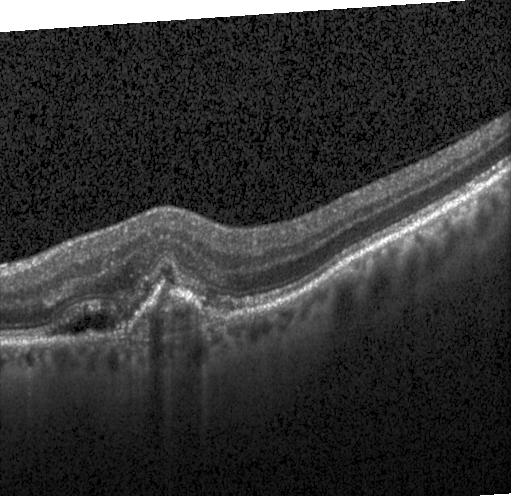

Heidelberg Spectralis · optical coherence tomography scan
A choroidal neovascular membrane.